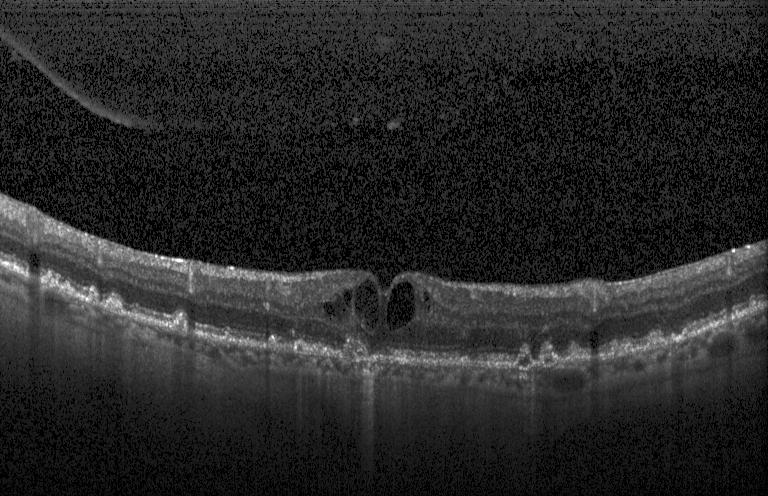

Spectral-domain optical coherence tomography; retinal OCT cross-section; macular scan
Finding: choroidal neovascularization.